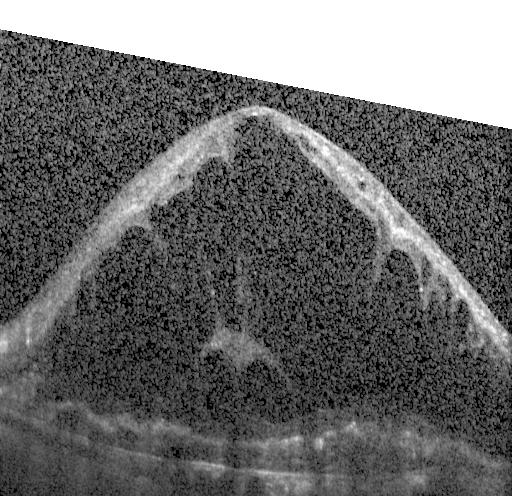

Optical coherence tomography scan.
Dx: a choroidal neovascular membrane.